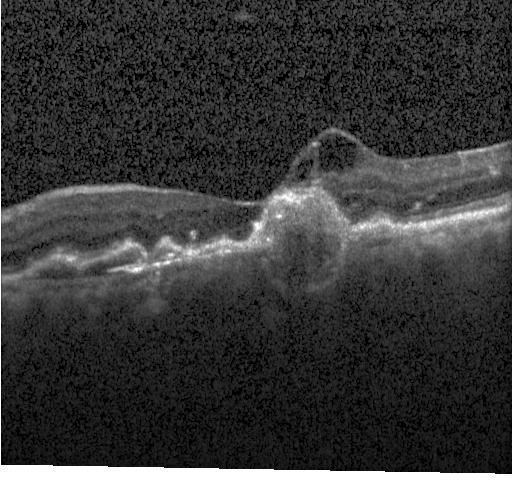 Retinal OCT B-scan. The scan shows choroidal neovascularization.